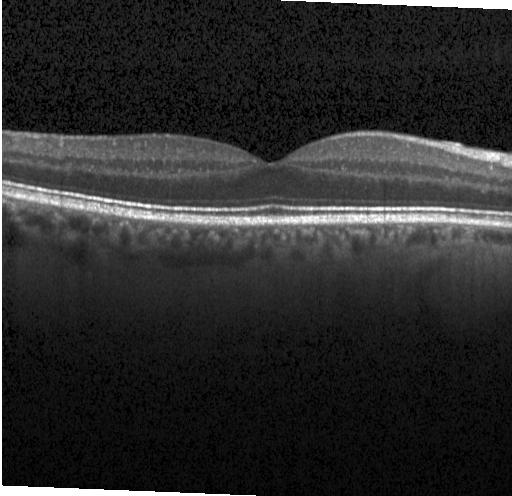
Optical coherence tomography B-scan.
This B-scan demonstrates no evidence of choroidal neovascularization, diabetic macular edema, or drusen.